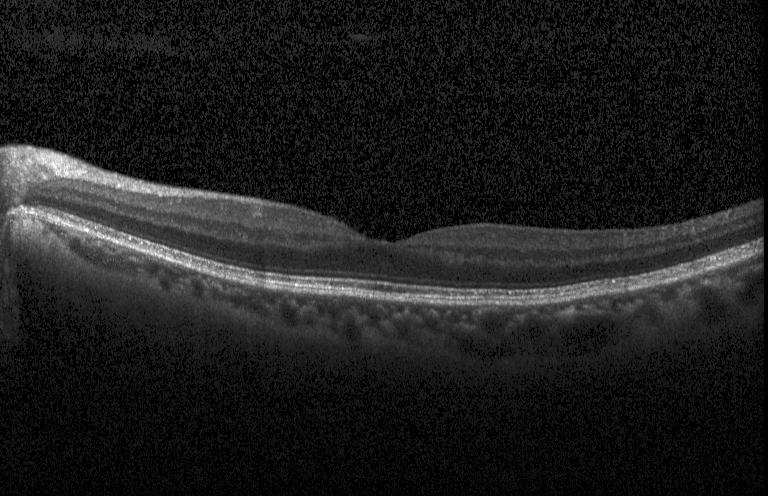 Spectral-domain OCT B-scan: no evidence of choroidal neovascularization, diabetic macular edema, or drusen.